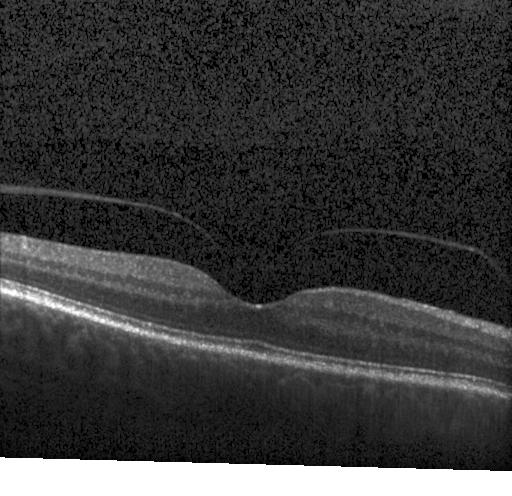 Optical coherence tomography scan · through the macula · spectral-domain OCT · Heidelberg Spectralis OCT system. Dx: no evidence of CNV, DME, or drusen.